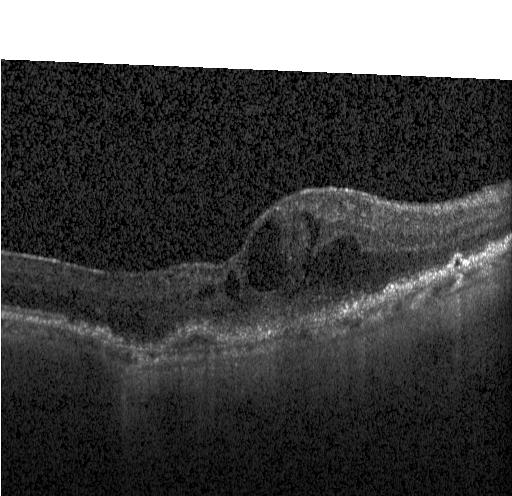

Spectral-domain optical coherence tomography; horizontal scan through the fovea; OCT B-scan; acquired on a Heidelberg Spectralis — Finding: a choroidal neovascular membrane.